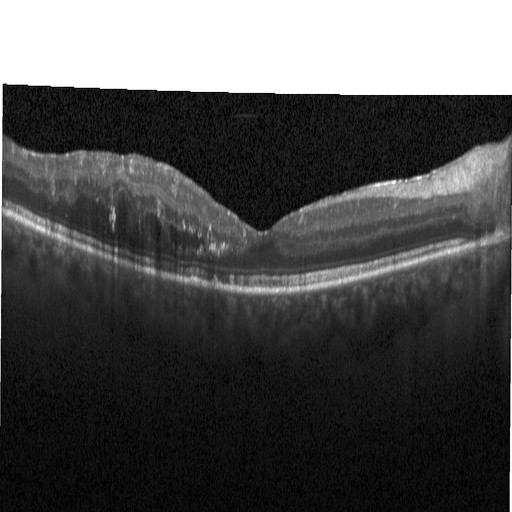 OCT B-scan; instrument: Heidelberg Spectralis; horizontal scan through the fovea.
Impression: diabetic macular edema (DME).